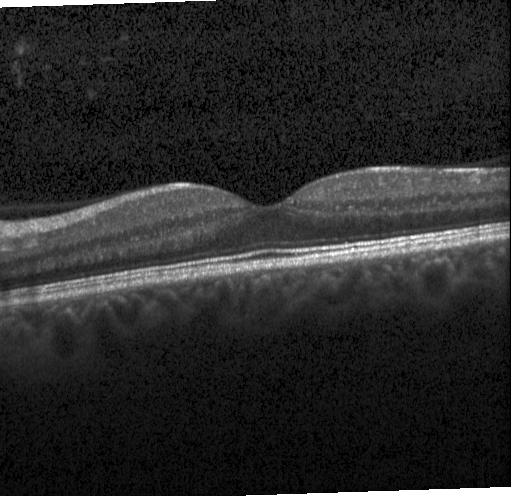

Heidelberg Spectralis, OCT B-scan, through the macula.
Finding: neither CNV, DME, nor drusen.